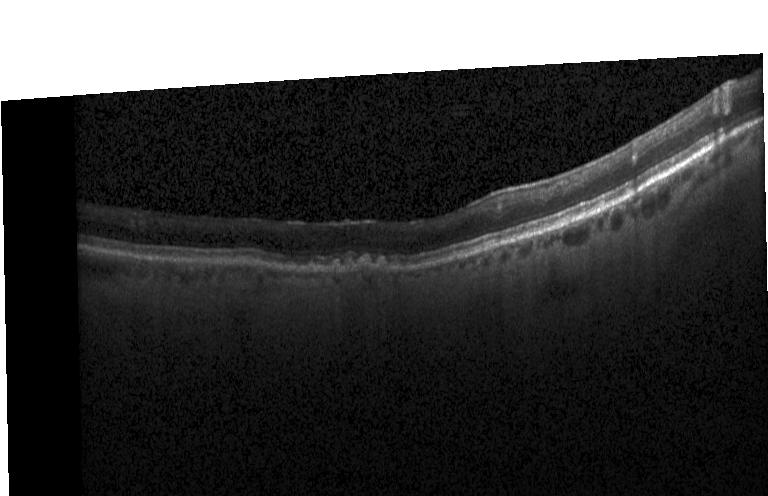
Retinal OCT cross-section showing multiple drusen.